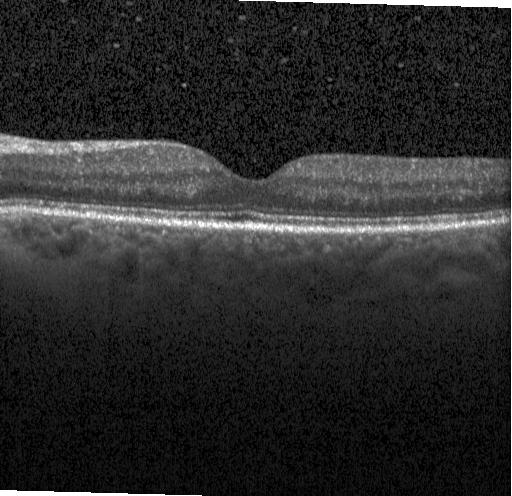

Dx: no evidence of CNV, DME, or drusen.